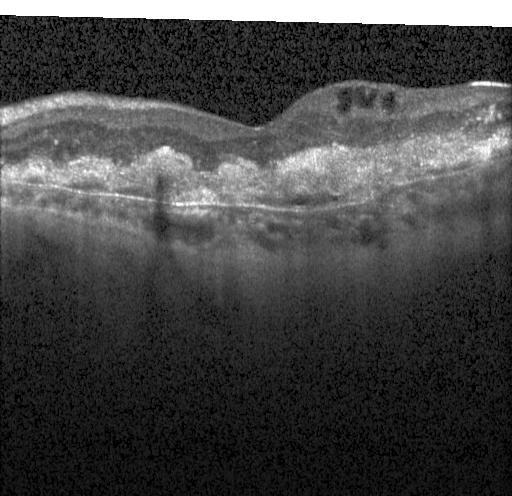 Optical coherence tomography B-scan; centered on the fovea
Diagnosis: a choroidal neovascular membrane.